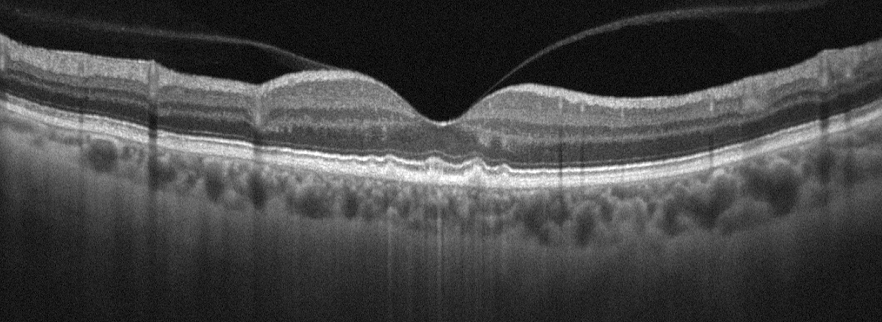 Optovue Avanti RTVue XR · OCT B-scan — Diagnosis: age-related macular degeneration.